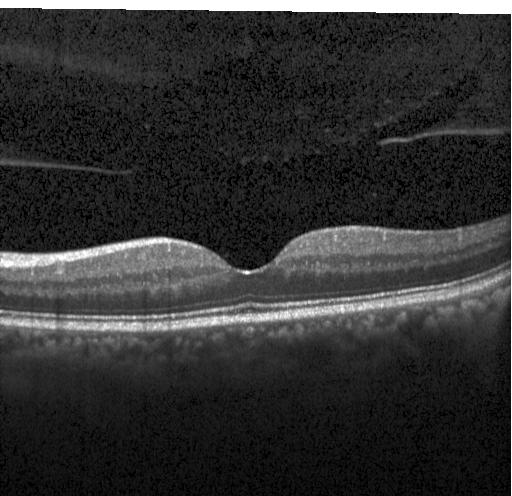 Macular scan; retinal OCT B-scan.
Impression: neither choroidal neovascularization, diabetic macular edema, nor drusen.